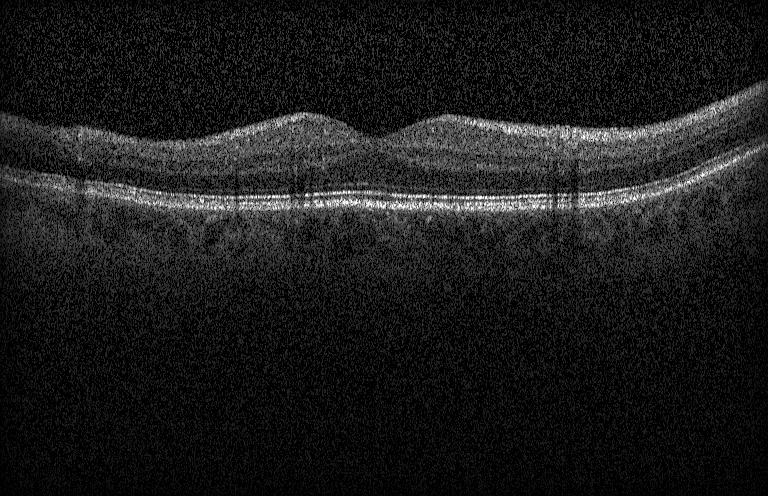
OCT line scan, centered on the fovea.
Finding: no choroidal neovascularization, no diabetic macular edema, and no drusen.